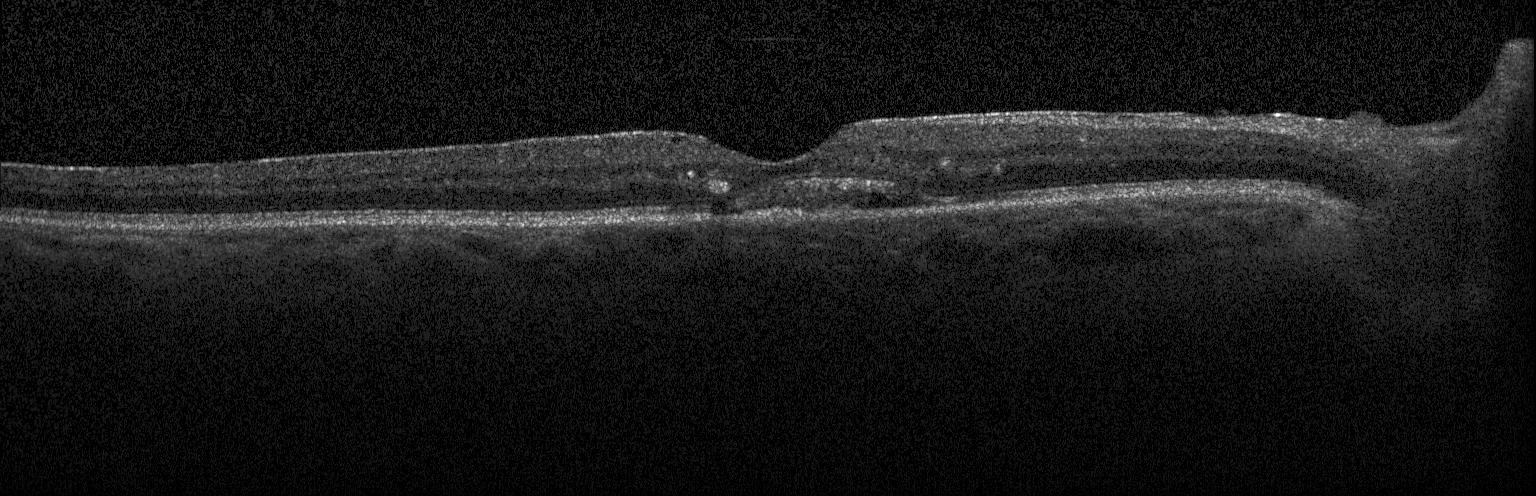
Retinal OCT cross-section, Heidelberg Spectralis OCT system, SD-OCT
Finding: CNV.